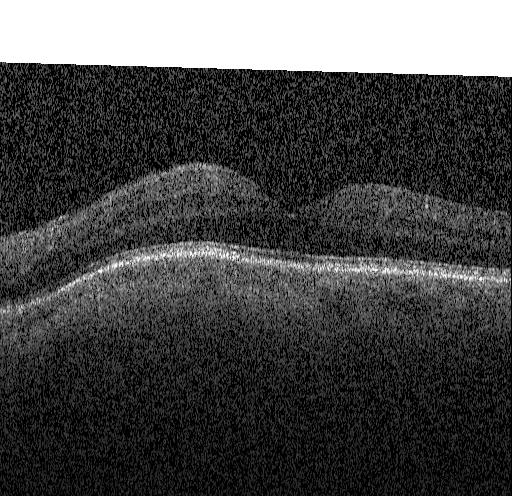
Heidelberg Spectralis · horizontal scan through the fovea · spectral-domain optical coherence tomography · OCT line scan
Finding: neither choroidal neovascularization, diabetic macular edema, nor drusen.